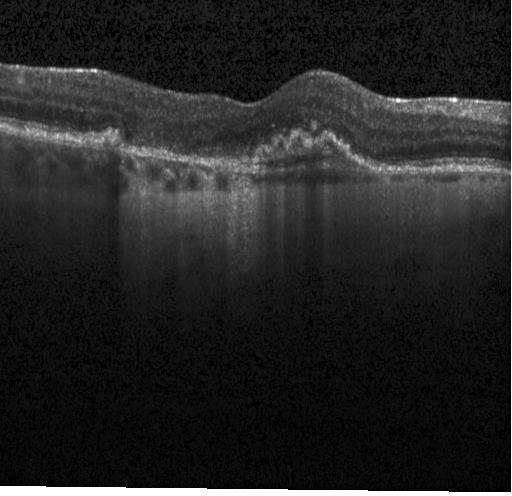 Impression: choroidal neovascularization.